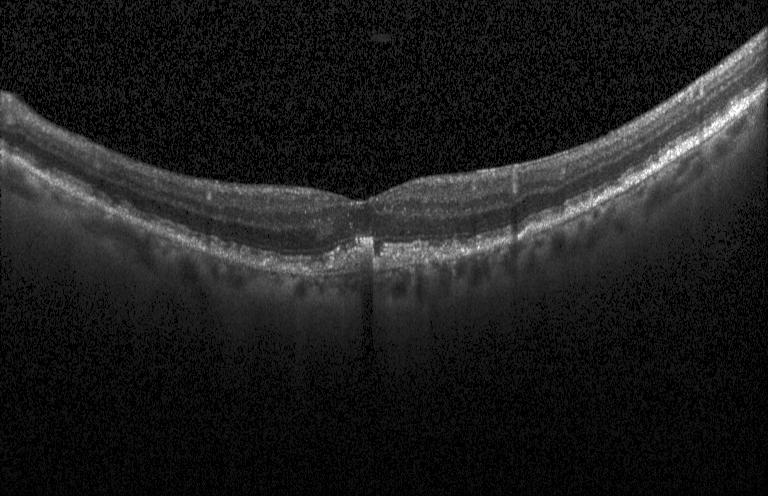

Horizontal scan through the fovea. OCT line scan
Dx: a choroidal neovascular membrane.